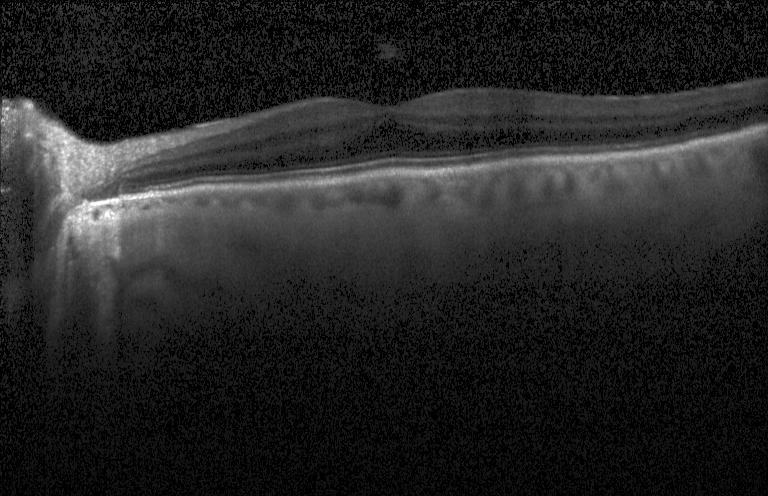
Macular OCT demonstrating no choroidal neovascularization, diabetic macular edema, or drusen.